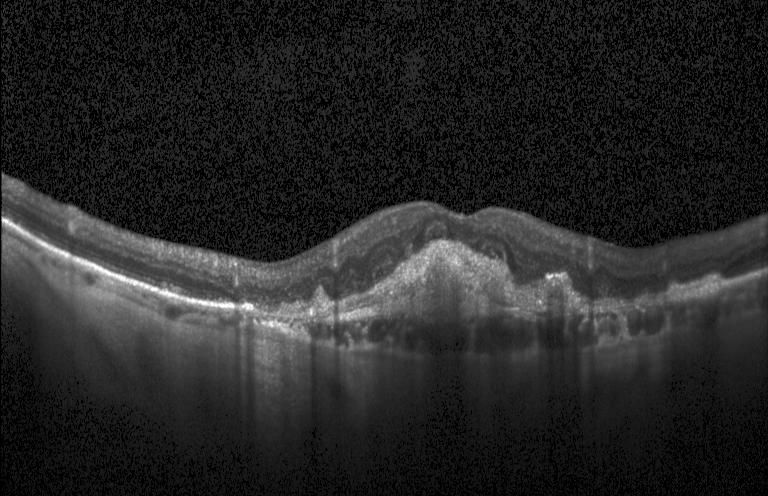
Instrument: Heidelberg Spectralis, through the macula, retinal OCT cross-section.
Assessment: a choroidal neovascular membrane.